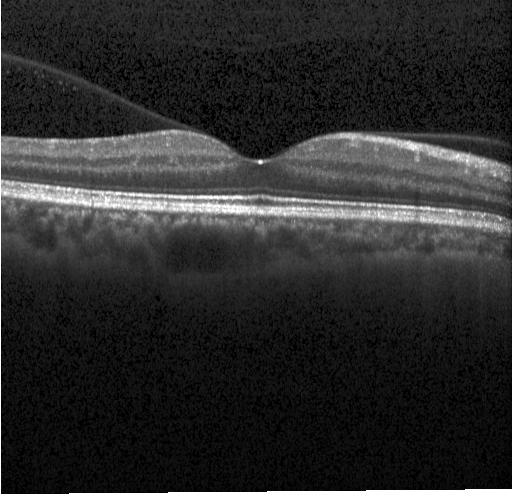

Heidelberg Spectralis OCT system · optical coherence tomography scan
Impression: no choroidal neovascularization, no diabetic macular edema, and no drusen.